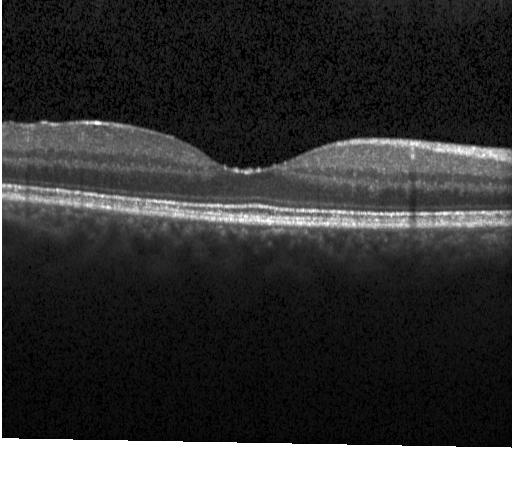

Heidelberg Spectralis · spectral-domain OCT · OCT line scan — No evidence of CNV, DME, or drusen.